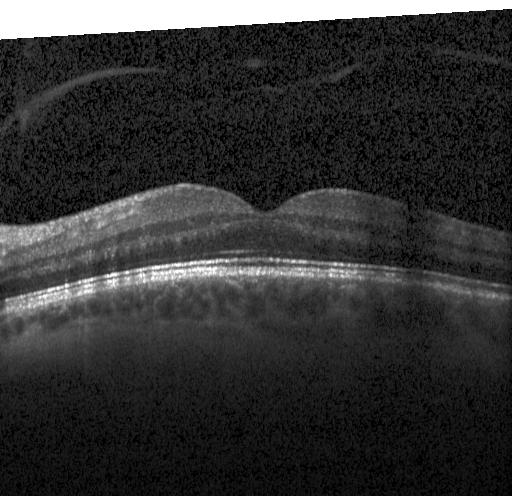
Instrument: Heidelberg Spectralis · retinal OCT B-scan — Finding: neither CNV, DME, nor drusen.